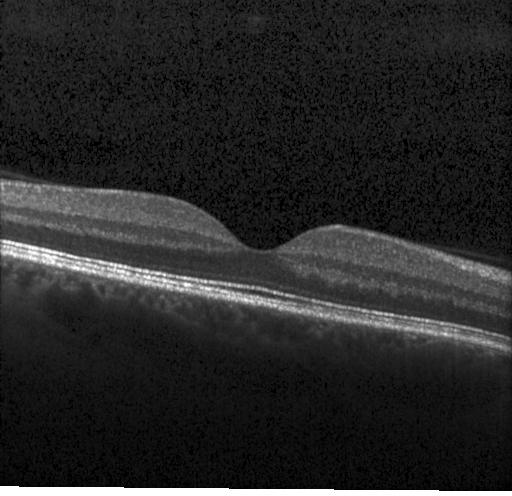
Retinal OCT cross-section showing neither choroidal neovascularization, diabetic macular edema, nor drusen.